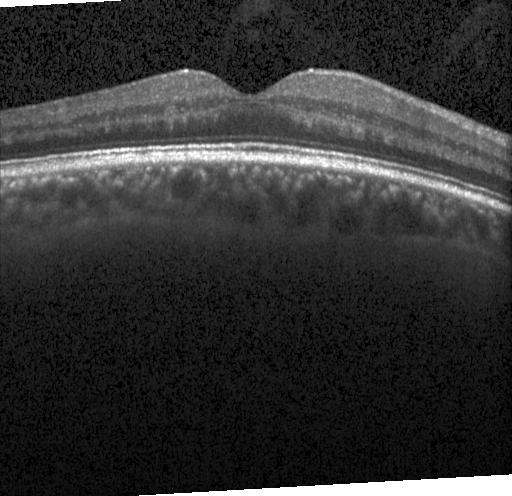
Optical coherence tomography B-scan — Macular OCT: no evidence of choroidal neovascularization, diabetic macular edema, or drusen.